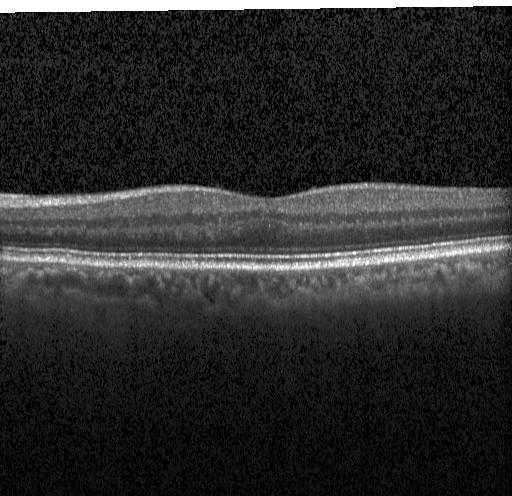

Spectral-domain optical coherence tomography, acquired on a Heidelberg Spectralis, retinal OCT B-scan
Macular OCT: neither choroidal neovascularization, diabetic macular edema, nor drusen.